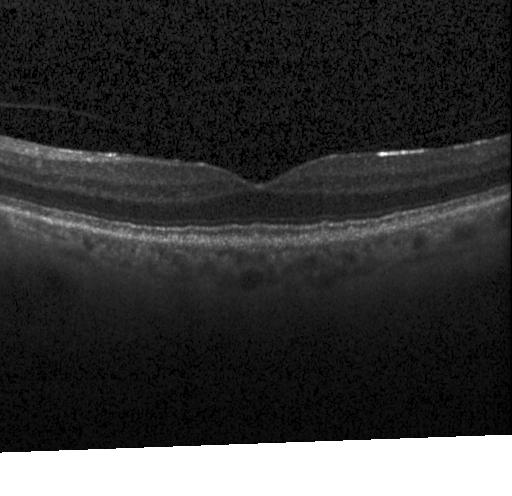

Retinal OCT cross-section, spectral-domain optical coherence tomography, fovea-centered, acquired on a Heidelberg Spectralis. Drusen.